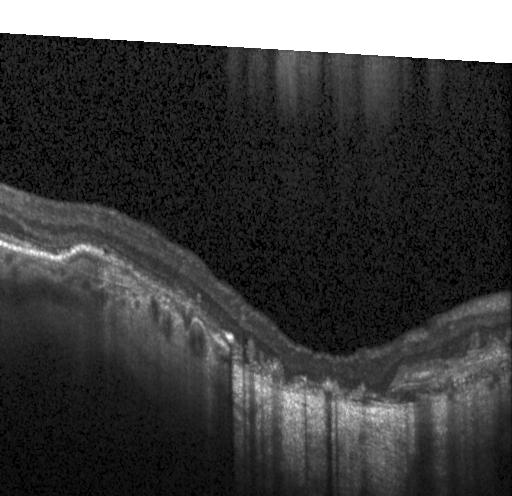
Through the macula · spectral-domain optical coherence tomography · OCT B-scan · Heidelberg Spectralis
The scan shows a choroidal neovascular membrane.